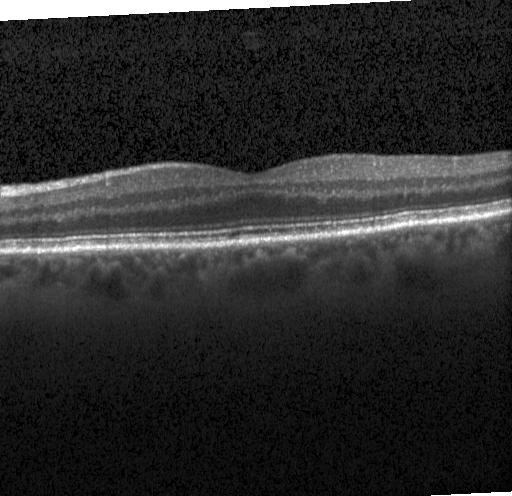 Macular OCT: no CNV, DME, or drusen.